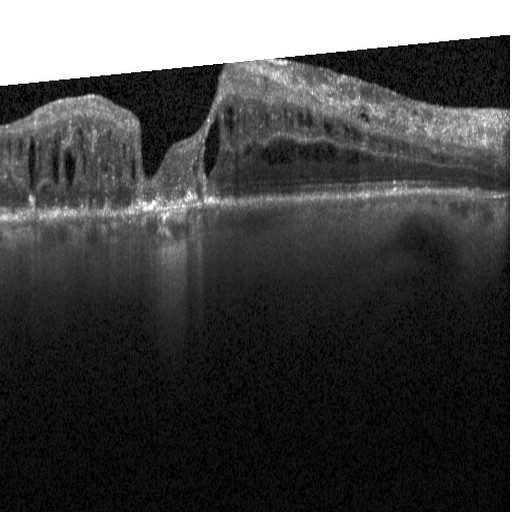

OCT line scan, Heidelberg Spectralis OCT system.
This B-scan demonstrates diabetic macular edema (DME).